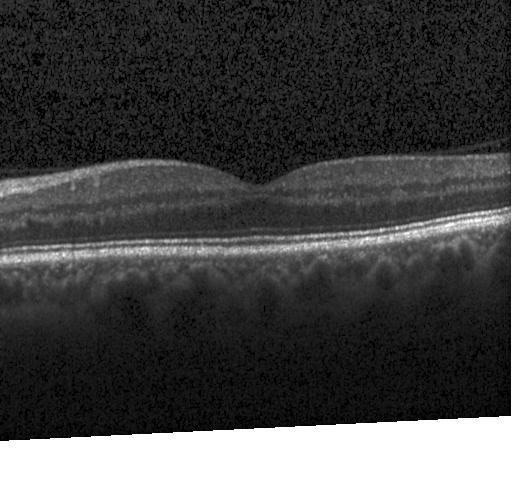

Spectral-domain OCT B-scan: no evidence of choroidal neovascularization, diabetic macular edema, or drusen.